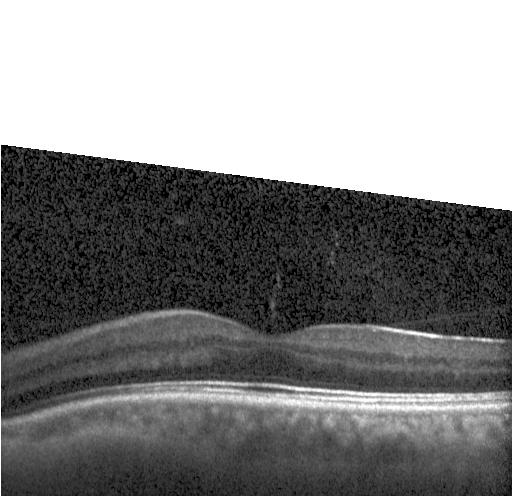

OCT scan showing no CNV, DME, or drusen.